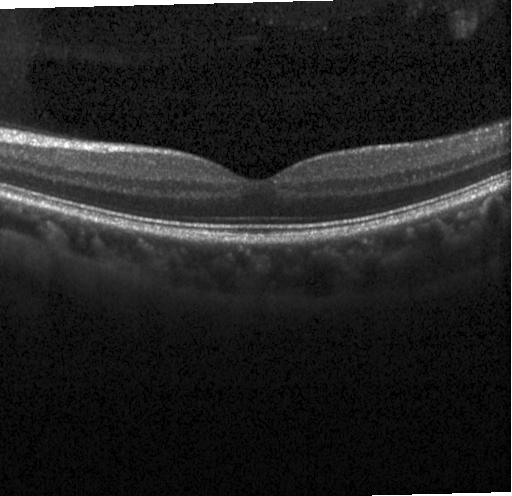

Macular scan · Heidelberg Spectralis · spectral-domain OCT · retinal OCT cross-section — Finding: no choroidal neovascularization, no diabetic macular edema, and no drusen.